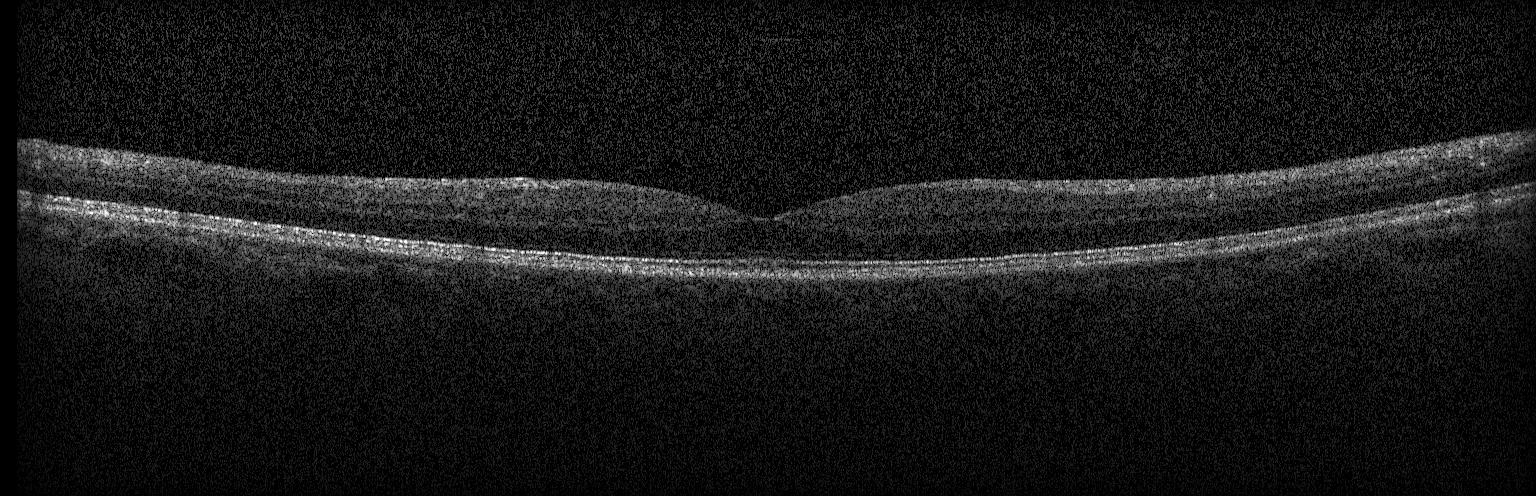

Macular OCT: no CNV, DME, or drusen.